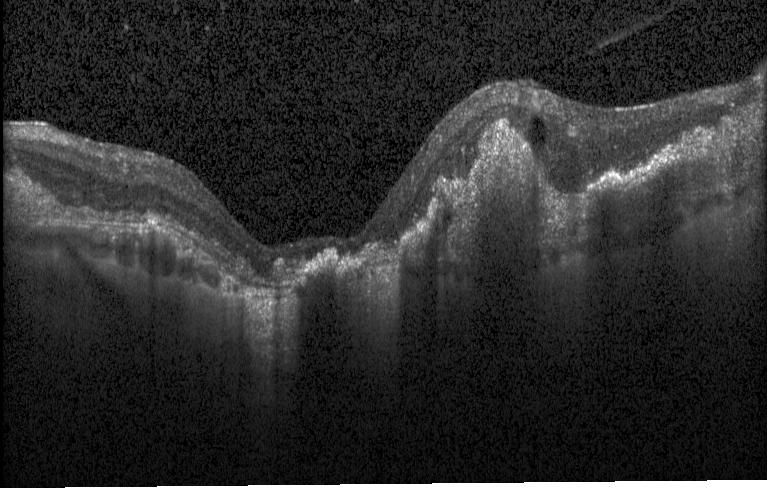
Spectral-domain OCT B-scan: a choroidal neovascular membrane.